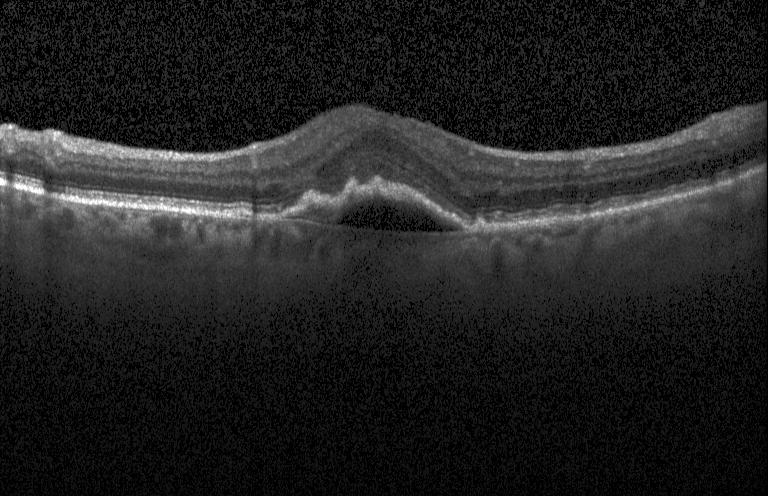 Macular OCT: choroidal neovascularization.